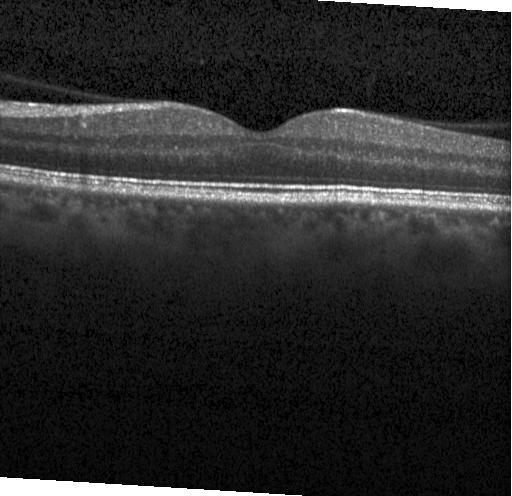

Optical coherence tomography B-scan — Finding: neither choroidal neovascularization, diabetic macular edema, nor drusen.